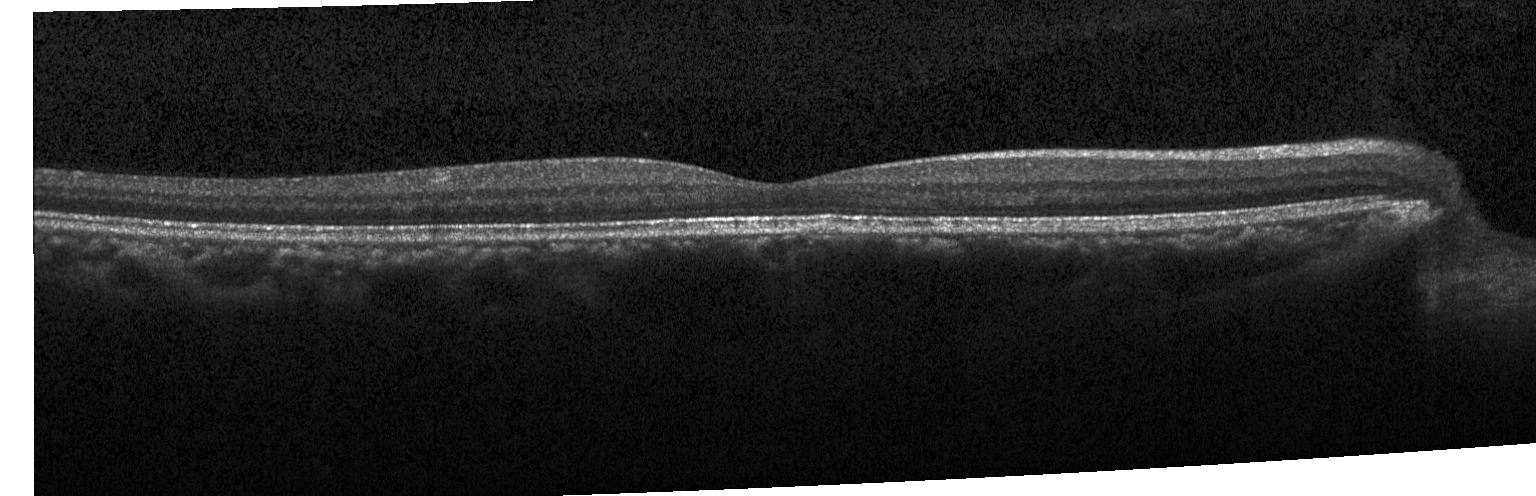
Impression: no choroidal neovascularization, diabetic macular edema, or drusen.